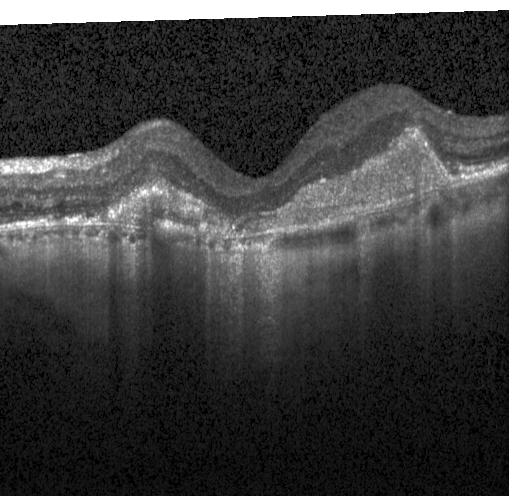
Macular scan, instrument: Heidelberg Spectralis, spectral-domain OCT, retinal OCT B-scan — Diagnosis: a choroidal neovascular membrane.